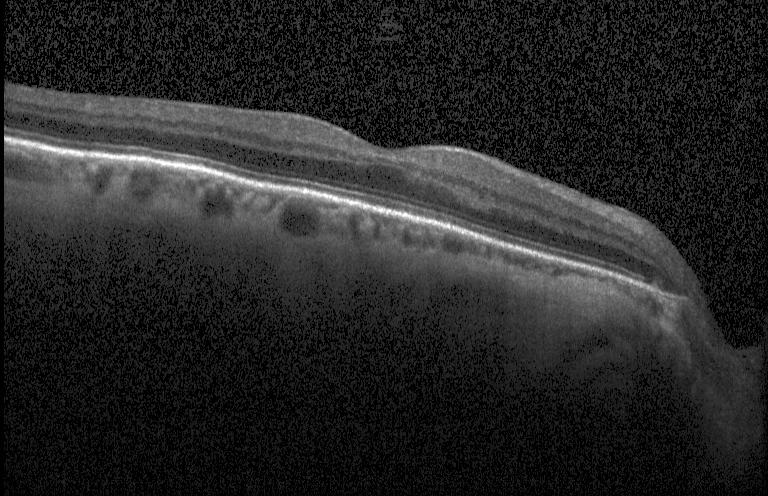
Retinal OCT B-scan. This B-scan demonstrates no choroidal neovascularization, diabetic macular edema, or drusen.